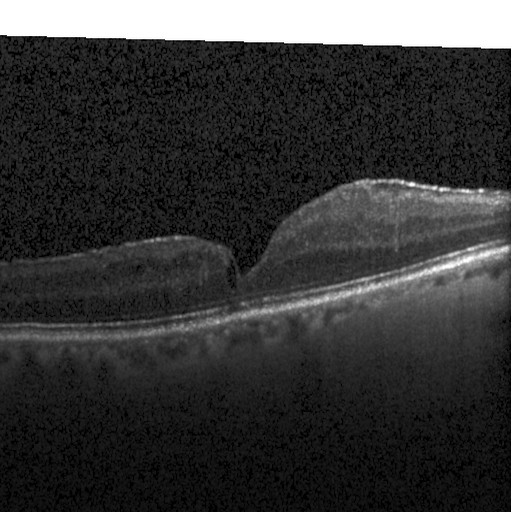 Heidelberg Spectralis OCT system · OCT B-scan.
Macular OCT: diabetic macular edema (DME).